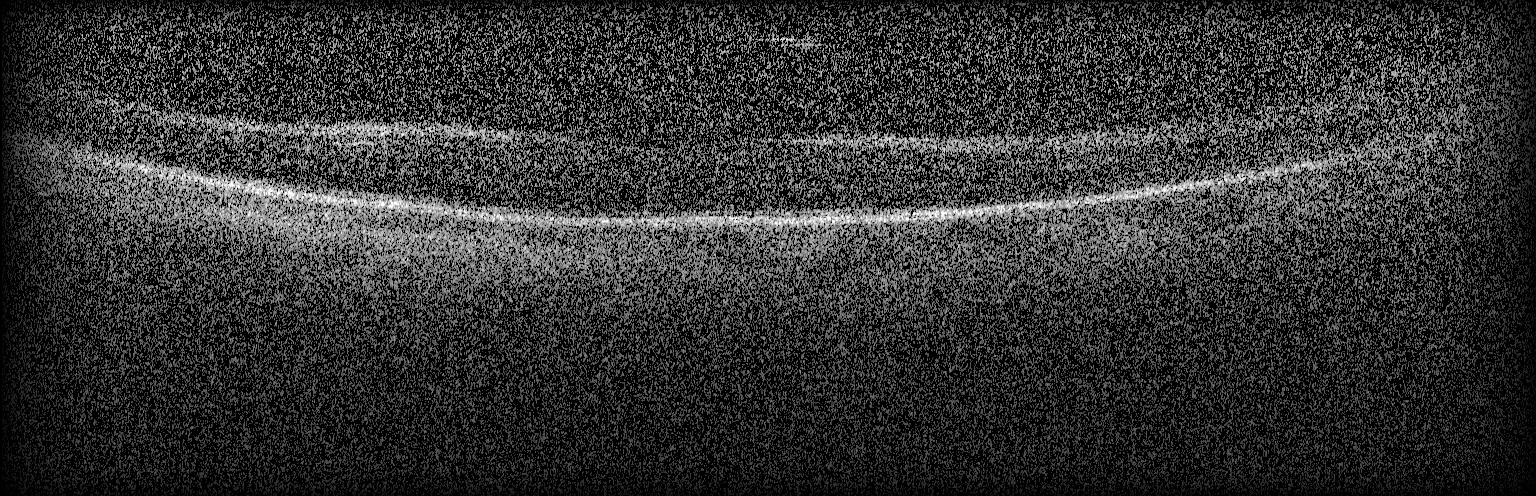 Optical coherence tomography B-scan.
Assessment: no choroidal neovascularization, diabetic macular edema, or drusen.